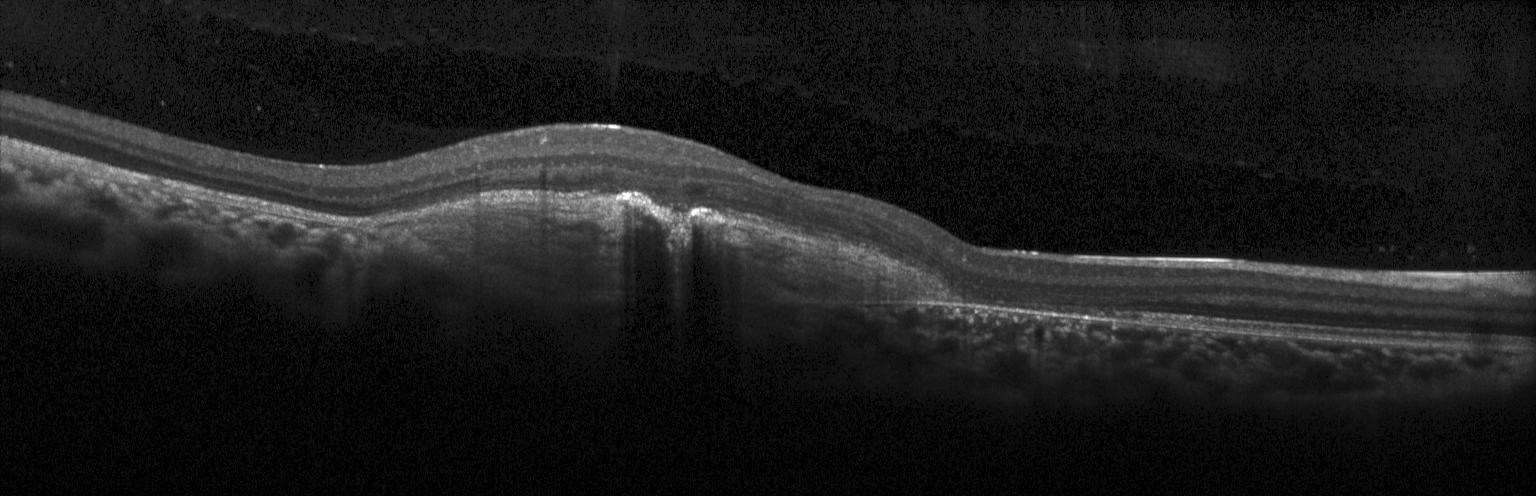

OCT line scan — Impression: CNV.